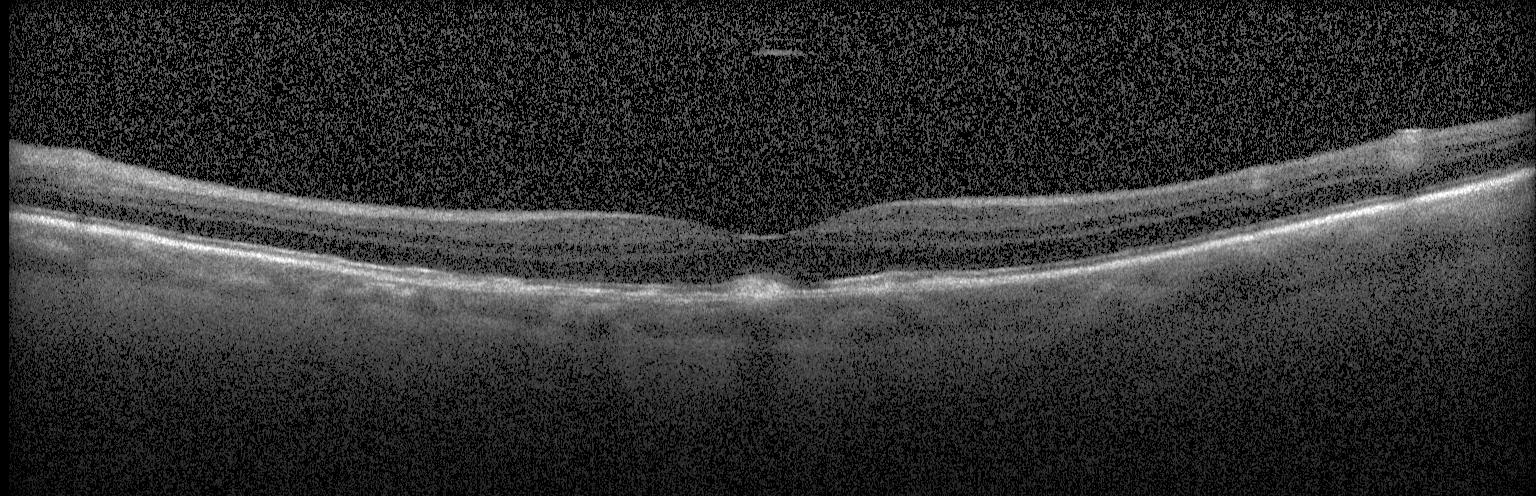

Optical coherence tomography scan, SD-OCT — OCT finding: choroidal neovascularization.